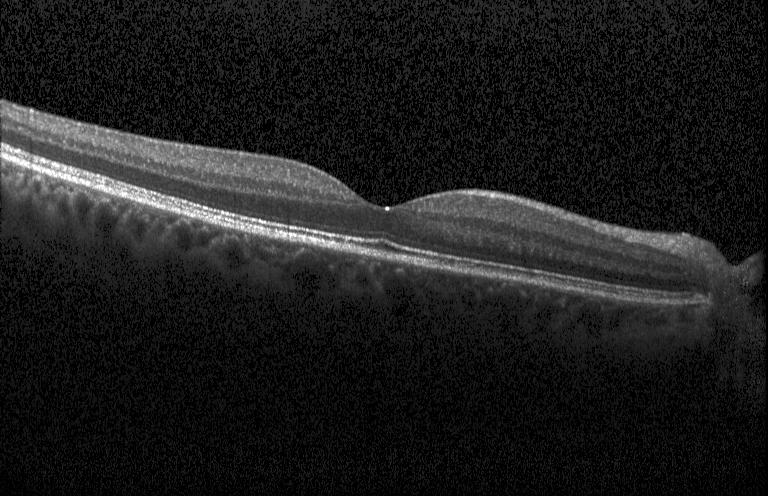
Retinal OCT B-scan
OCT finding: no choroidal neovascularization, no diabetic macular edema, and no drusen.